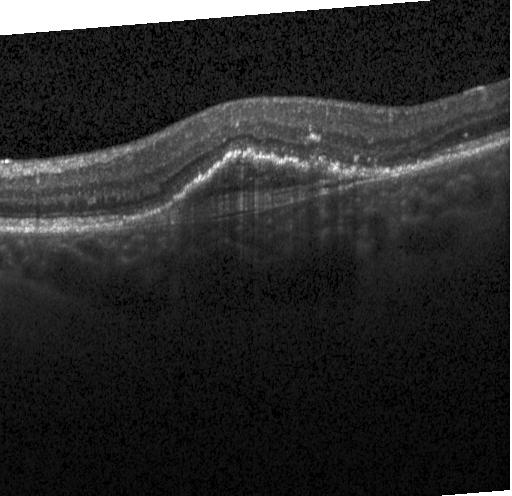

Impression: a choroidal neovascular membrane.